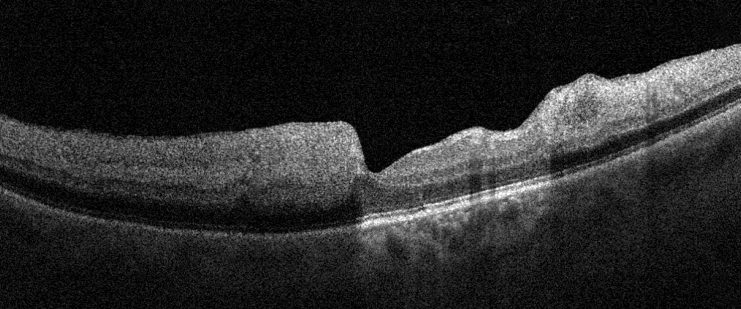
Through the macula; optical coherence tomography scan.
This B-scan demonstrates retinal artery occlusion.